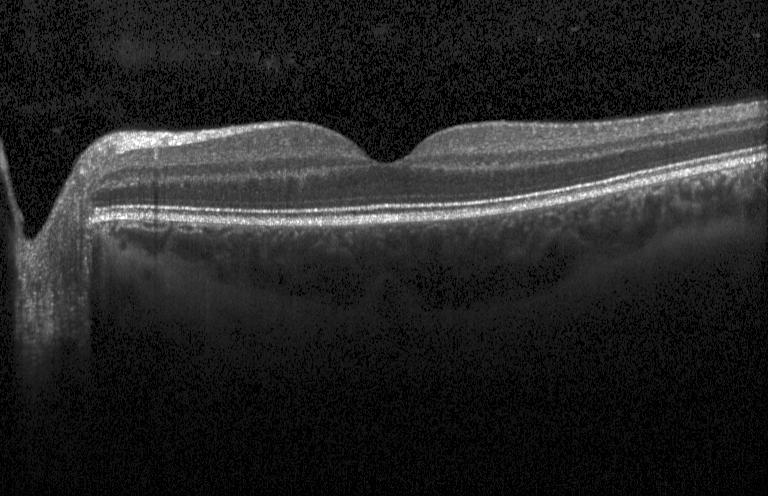
OCT line scan — OCT finding: no choroidal neovascularization, no diabetic macular edema, and no drusen.